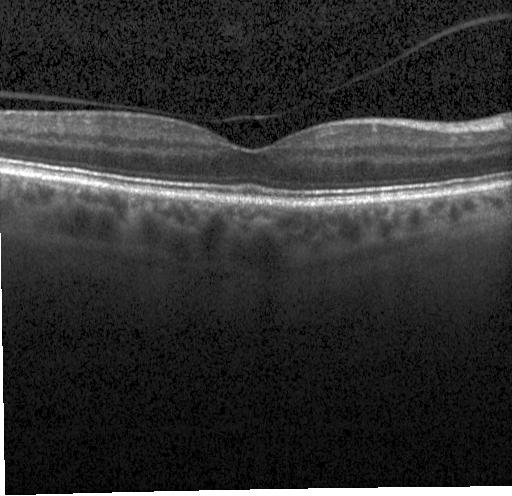

Impression: no choroidal neovascularization, no diabetic macular edema, and no drusen.